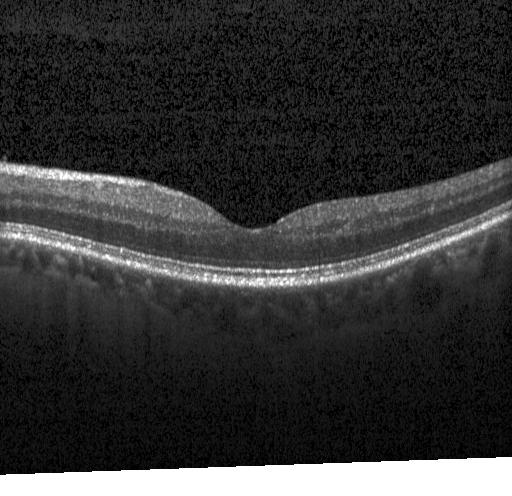
Retinal OCT cross-section — Macular OCT: no evidence of choroidal neovascularization, diabetic macular edema, or drusen.